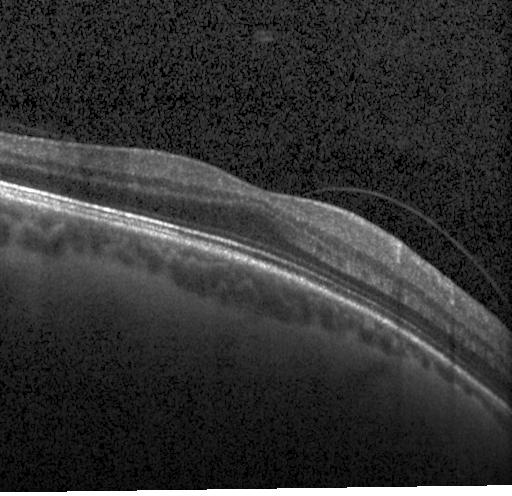

OCT finding: no choroidal neovascularization, no diabetic macular edema, and no drusen.